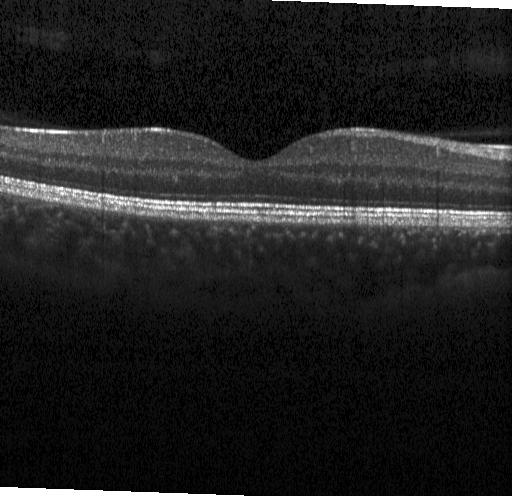
Spectral-domain optical coherence tomography; Heidelberg Spectralis OCT system; OCT line scan; macular scan.
Finding: neither choroidal neovascularization, diabetic macular edema, nor drusen.